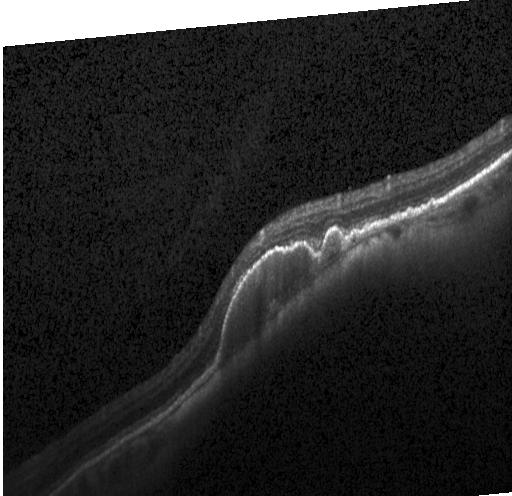 OCT B-scan showing CNV.